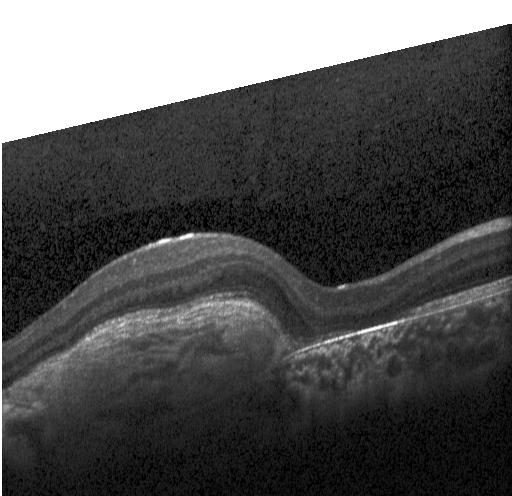

Impression: choroidal neovascularization (CNV).